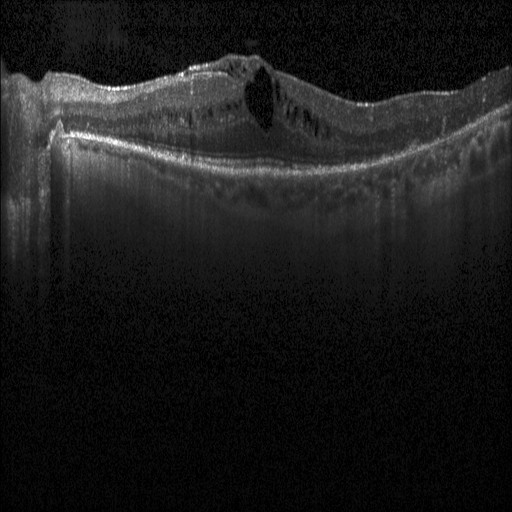
Retinal OCT B-scan · Heidelberg Spectralis OCT system
DME.